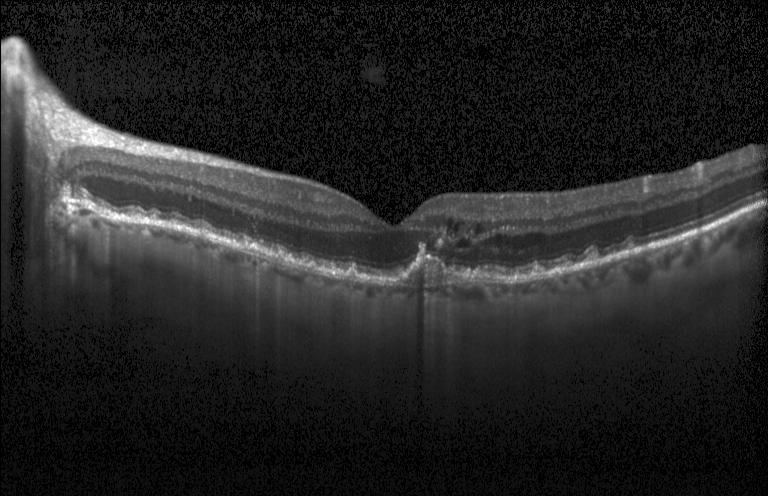
Macular scan · acquired on a Heidelberg Spectralis · SD-OCT · optical coherence tomography B-scan
Finding: a choroidal neovascular membrane.